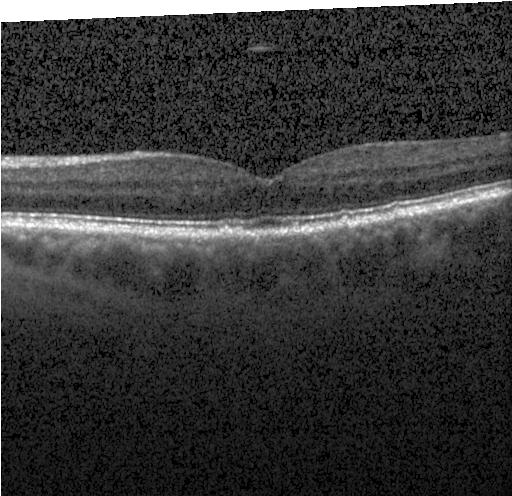
OCT scan showing sub-RPE drusenoid deposits.